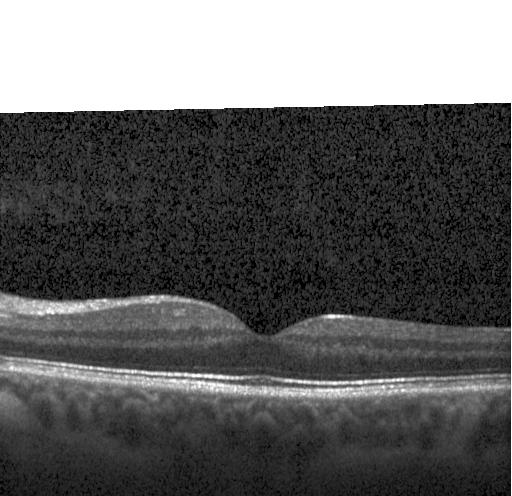

Macular OCT: no choroidal neovascularization, diabetic macular edema, or drusen.